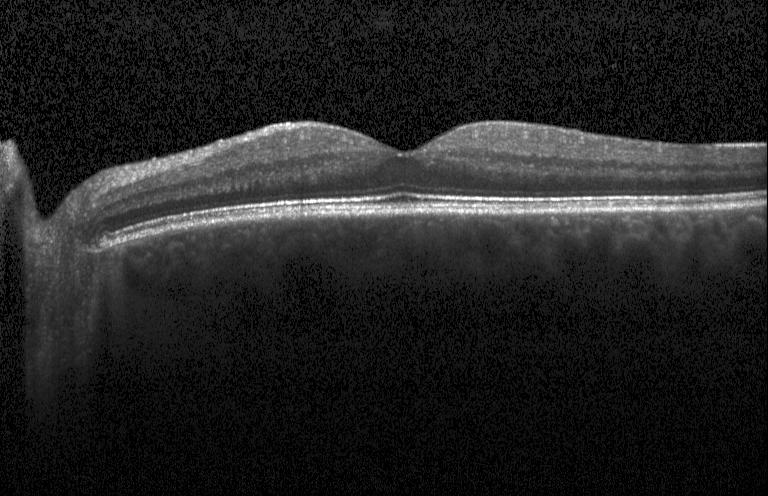 OCT B-scan showing no CNV, no DME, and no drusen.